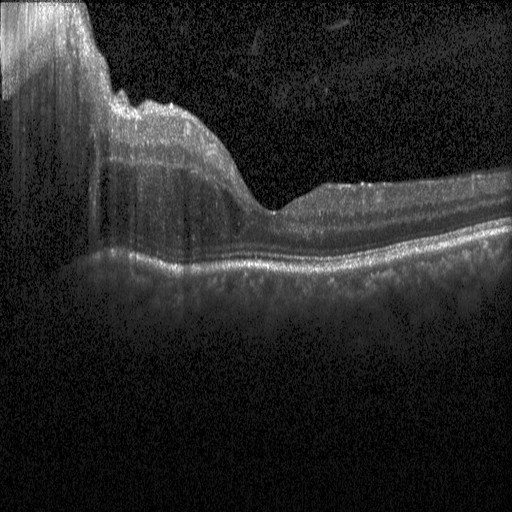
OCT B-scan.
OCT finding: DME.